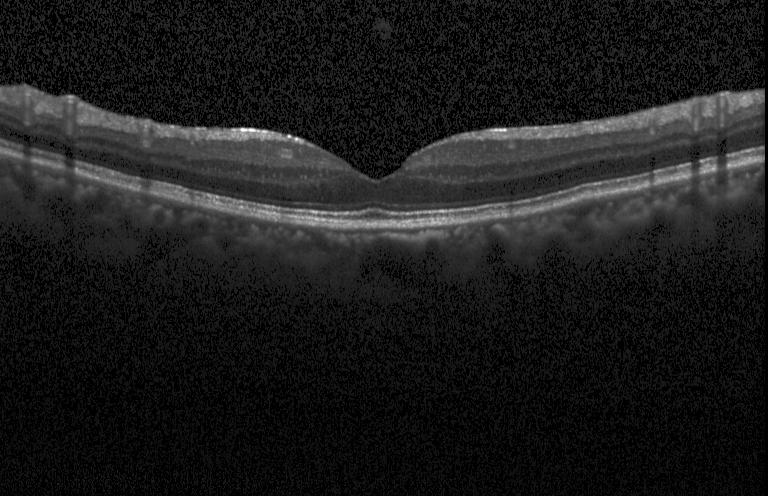 Impression: no evidence of choroidal neovascularization, diabetic macular edema, or drusen.